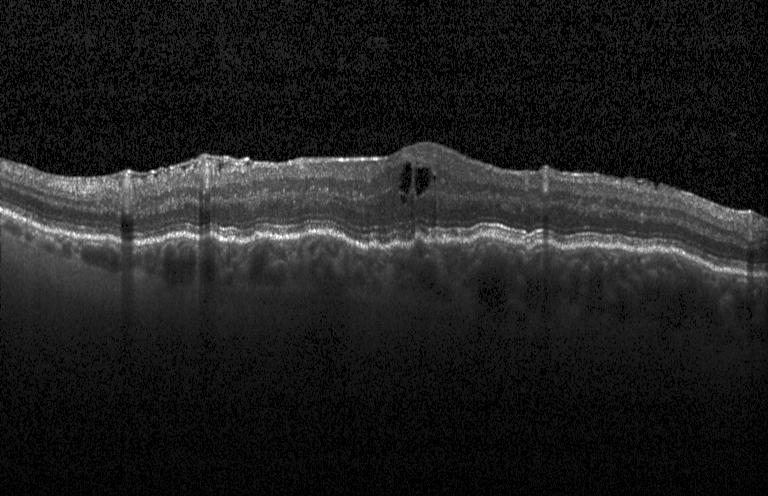 Centered on the fovea, spectral-domain optical coherence tomography, retinal OCT cross-section, Heidelberg Spectralis OCT system — Dx: diabetic macular edema (DME).